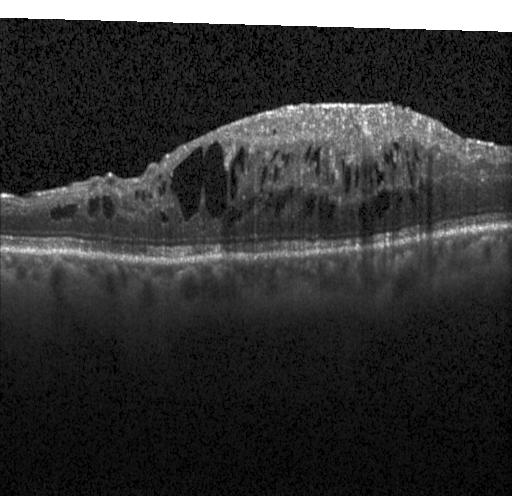
Centered on the fovea, retinal OCT B-scan, Heidelberg Spectralis OCT system.
Impression: diabetic macular edema (DME).